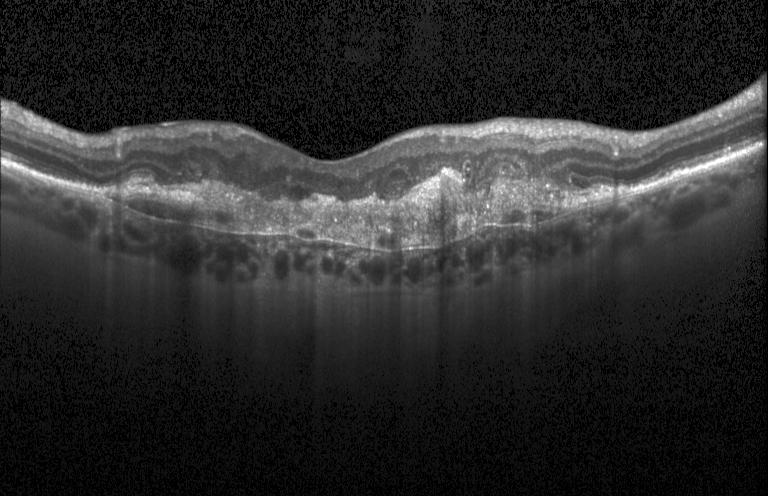

OCT line scan. Through the macula. This B-scan demonstrates choroidal neovascularization.